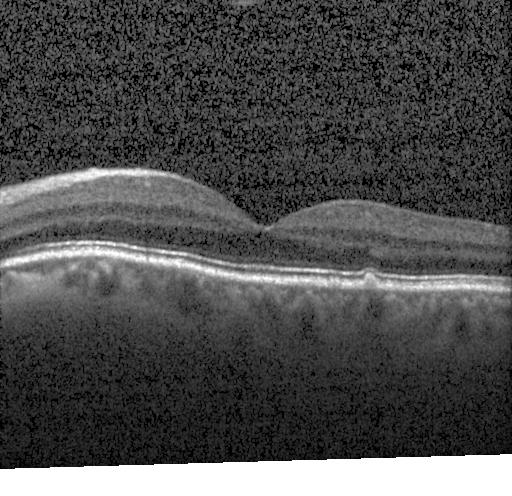
Spectral-domain OCT · OCT B-scan — Finding: multiple drusen.